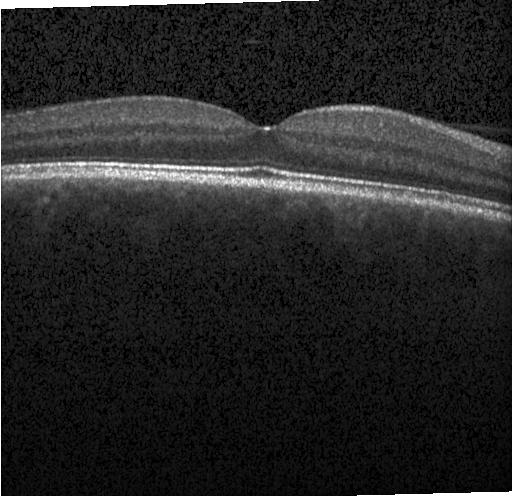
Heidelberg Spectralis · OCT line scan — Finding: neither choroidal neovascularization, diabetic macular edema, nor drusen.